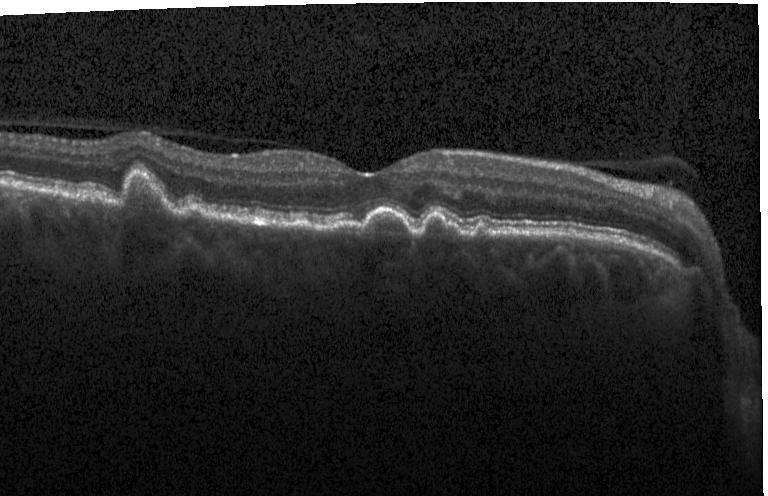

Impression: drusen.